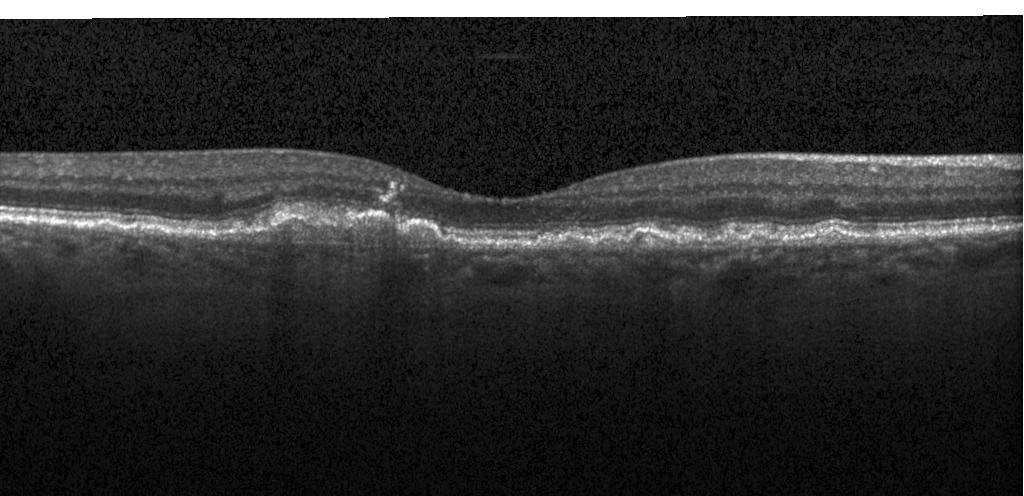 OCT line scan.
Diagnosis: choroidal neovascularization.